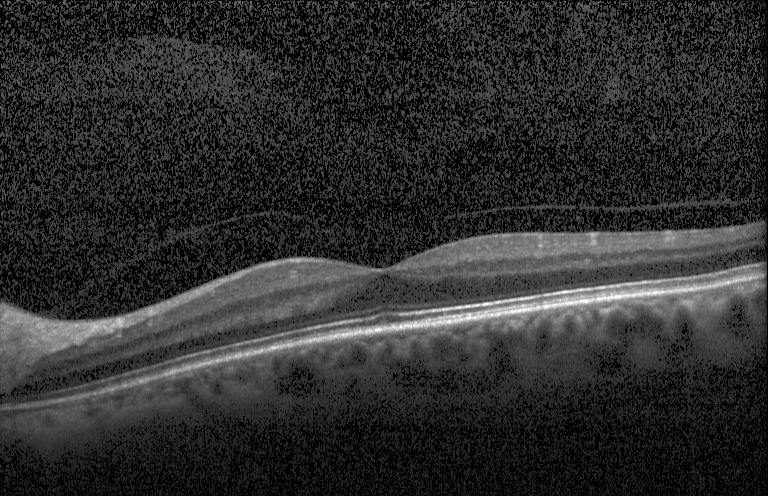 Impression: no CNV, DME, or drusen.